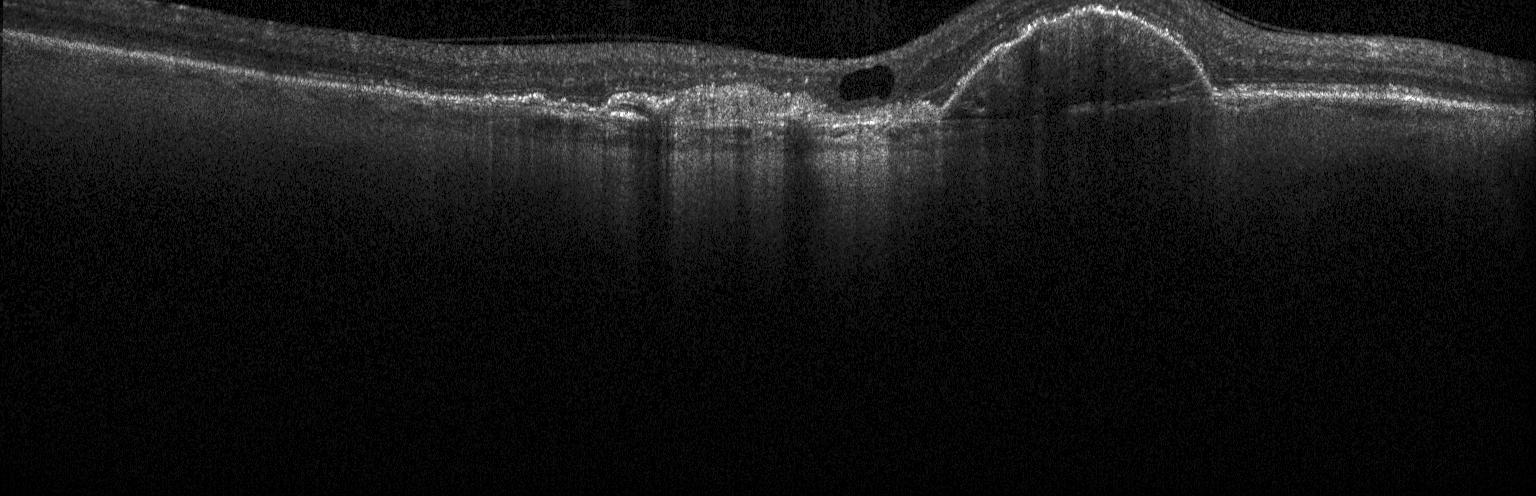

OCT line scan.
Choroidal neovascularization (CNV).